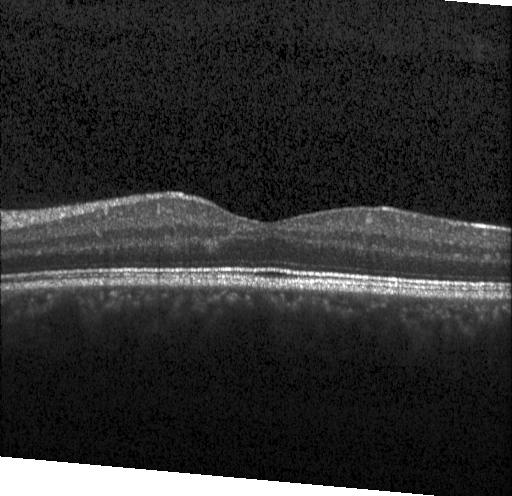 Diagnosis: neither choroidal neovascularization, diabetic macular edema, nor drusen.